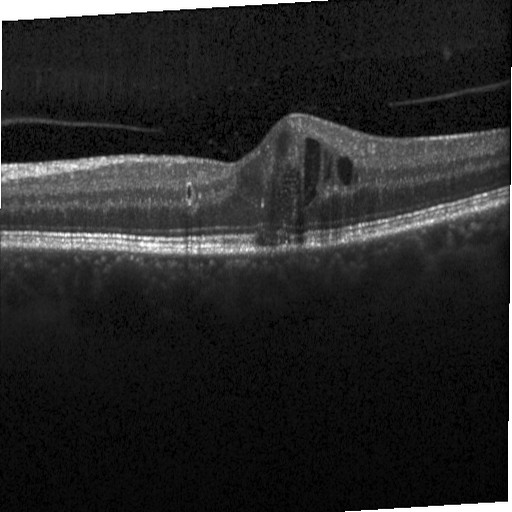 Instrument: Heidelberg Spectralis; OCT line scan; spectral-domain optical coherence tomography — Impression: diabetic macular edema (DME).